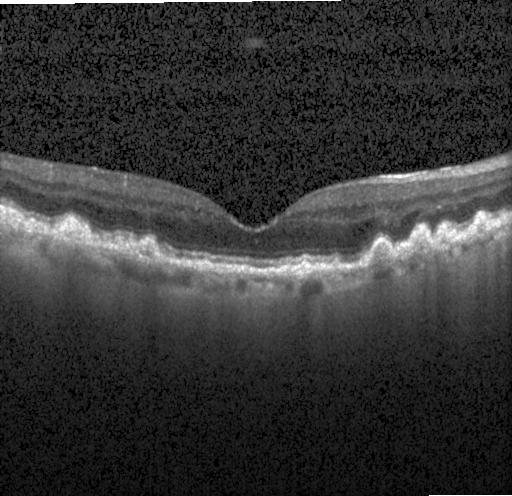 Centered on the fovea, instrument: Heidelberg Spectralis, spectral-domain OCT, optical coherence tomography B-scan — Diagnosis: sub-RPE drusenoid deposits.